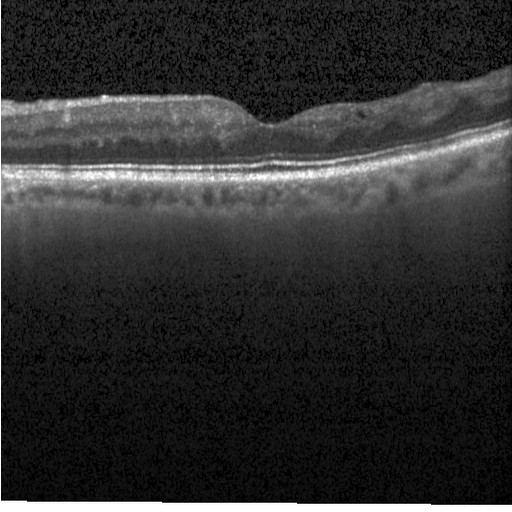

Spectral-domain OCT; OCT line scan.
Finding: diabetic macular edema.